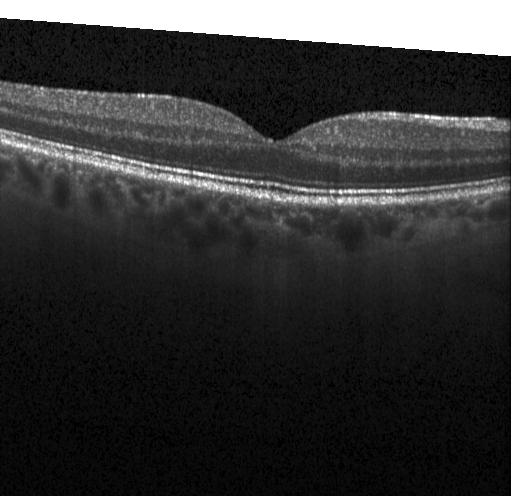 Impression: no evidence of CNV, DME, or drusen.